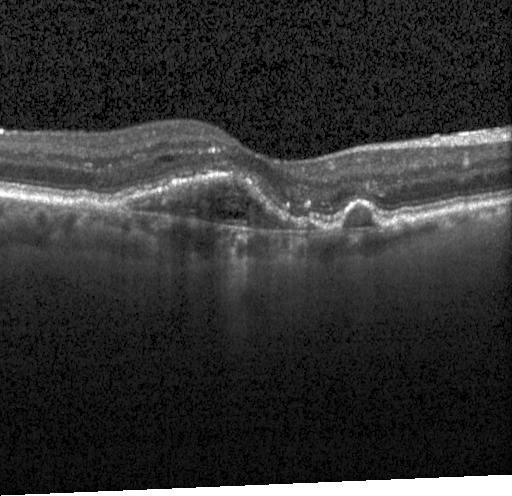
Assessment: a choroidal neovascular membrane.